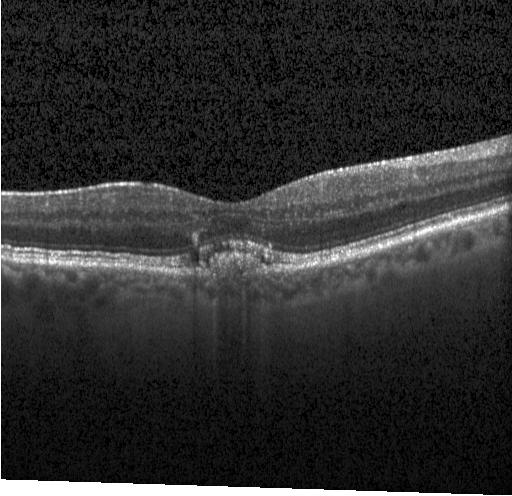

OCT B-scan.
The scan shows CNV.